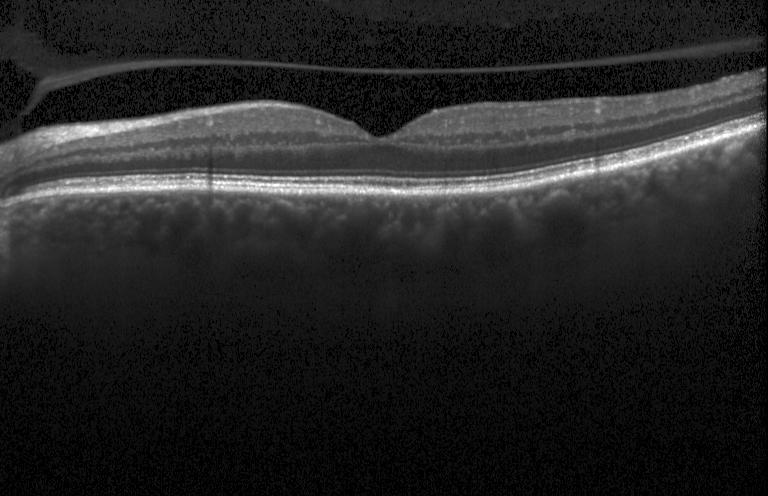
Fovea-centered · retinal OCT B-scan.
Assessment: neither CNV, DME, nor drusen.